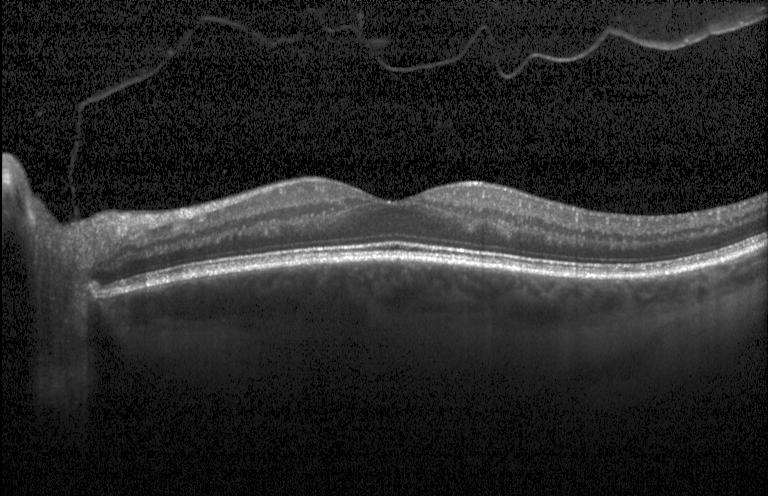
OCT line scan. Instrument: Heidelberg Spectralis. SD-OCT
The scan shows no choroidal neovascularization, diabetic macular edema, or drusen.